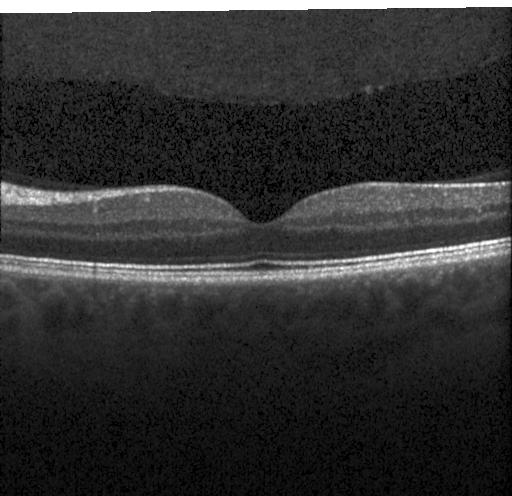
Retinal OCT cross-section showing neither choroidal neovascularization, diabetic macular edema, nor drusen.